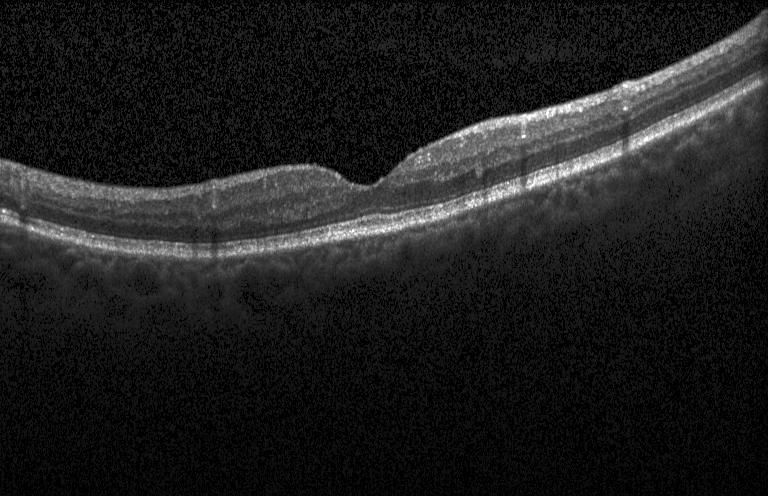

Impression: no choroidal neovascularization, diabetic macular edema, or drusen.